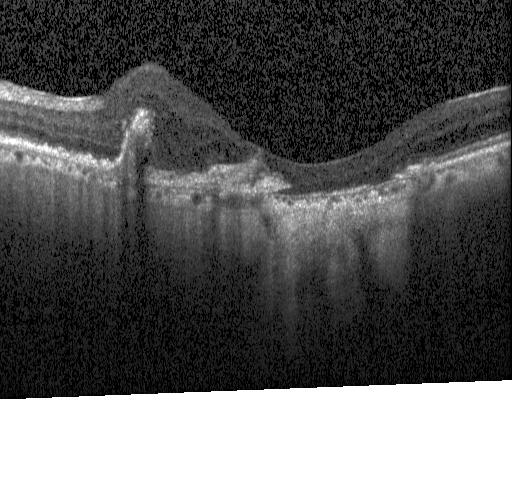 Through the macula. Acquired on a Heidelberg Spectralis. Retinal OCT B-scan. Spectral-domain optical coherence tomography — Finding: choroidal neovascularization.